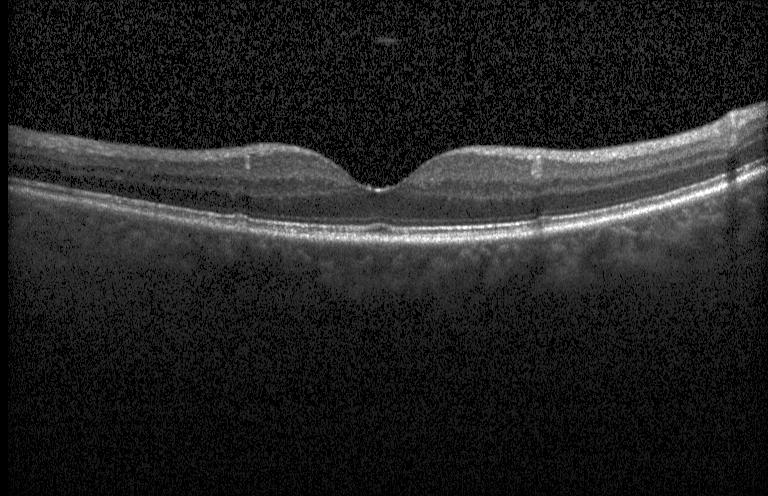

OCT B-scan showing no evidence of choroidal neovascularization, diabetic macular edema, or drusen.